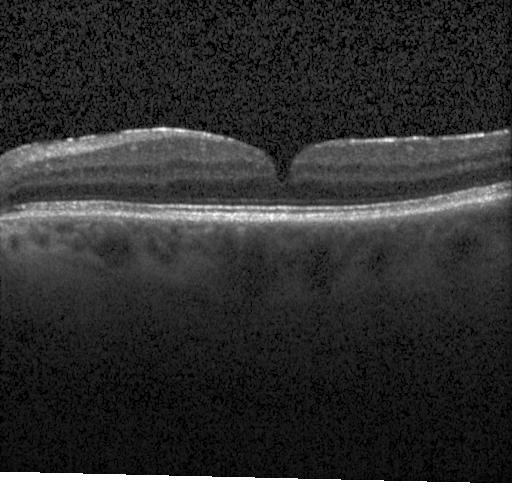 Retinal OCT cross-section showing no evidence of CNV, DME, or drusen.